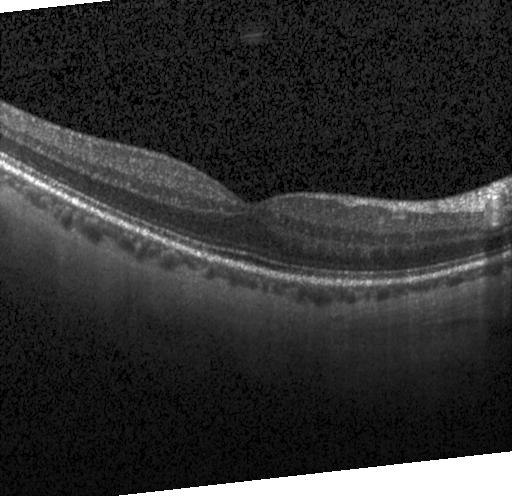 OCT B-scan
Impression: neither choroidal neovascularization, diabetic macular edema, nor drusen.